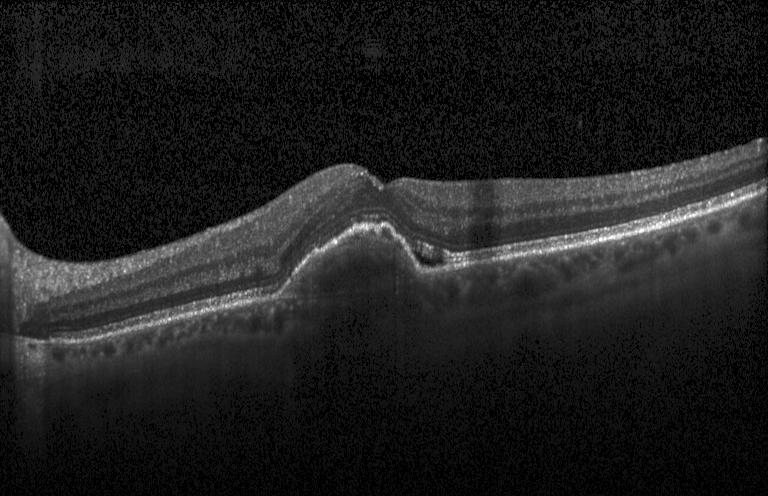
OCT line scan
Finding: choroidal neovascularization (CNV).